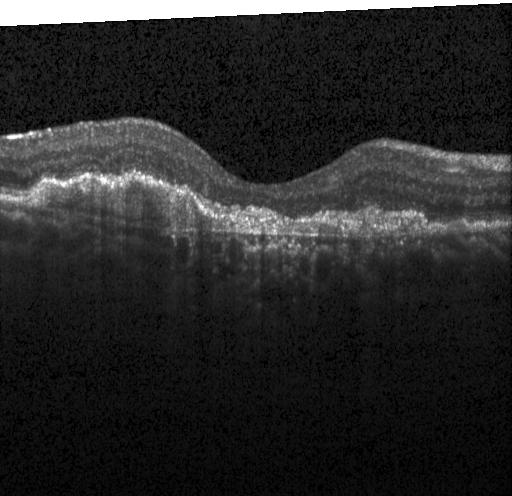
Fovea-centered; spectral-domain OCT; optical coherence tomography B-scan — Dx: a choroidal neovascular membrane.